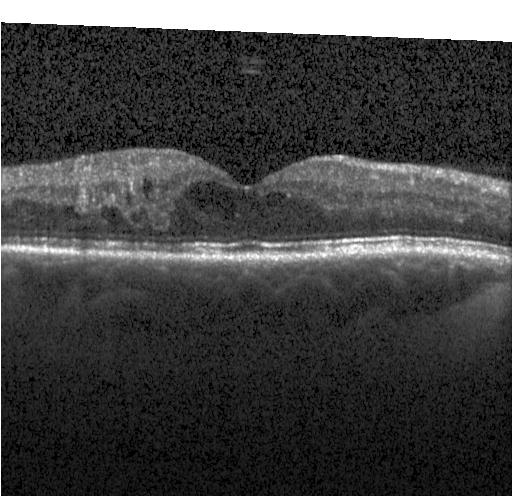

Impression: DME.